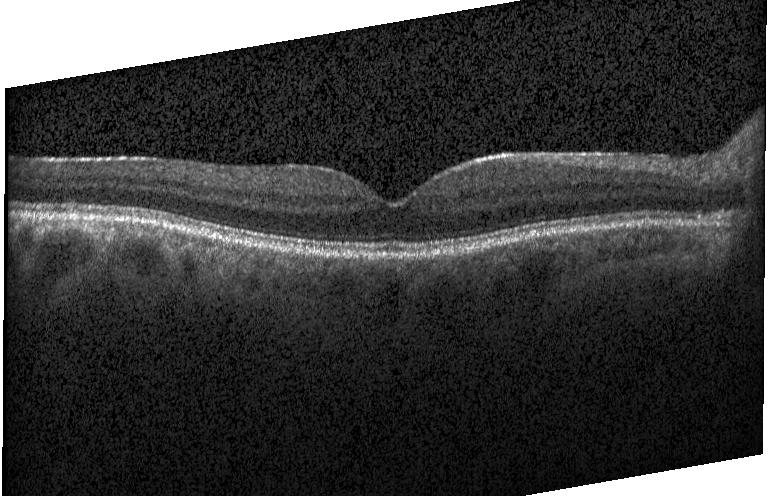
SD-OCT, through the macula, retinal OCT cross-section — The scan shows no CNV, no DME, and no drusen.